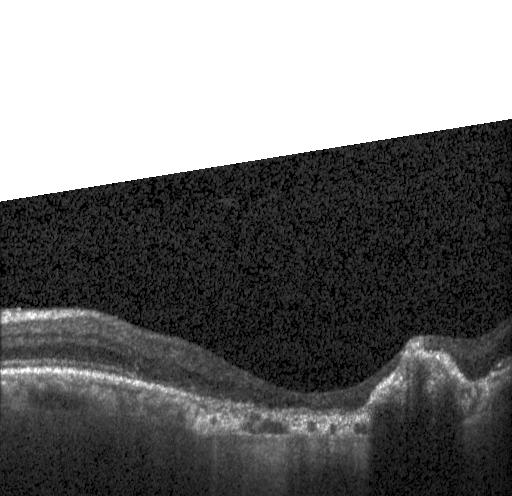 The scan shows a choroidal neovascular membrane.